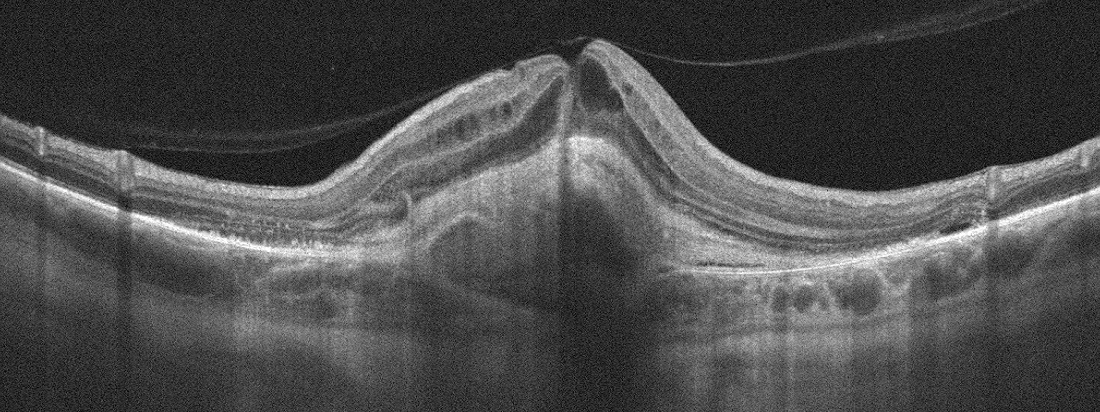

Acquired on an Optovue Avanti RTVue XR, macular scan, optical coherence tomography scan.
The scan shows age-related macular degeneration.